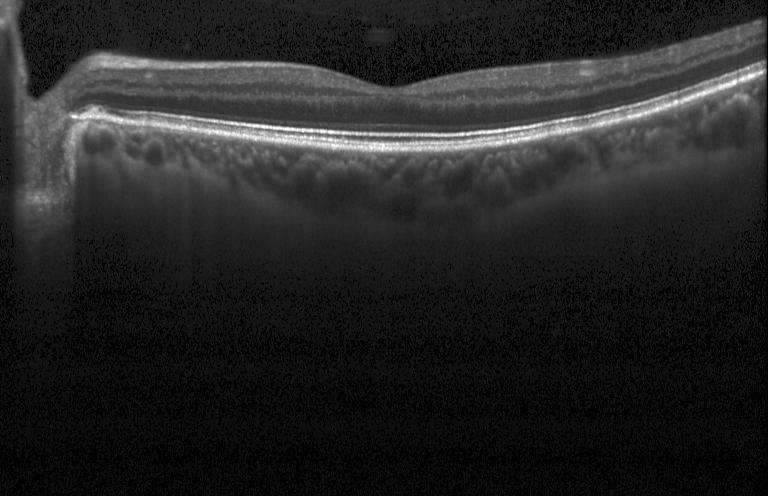

Diagnosis: no choroidal neovascularization, no diabetic macular edema, and no drusen.